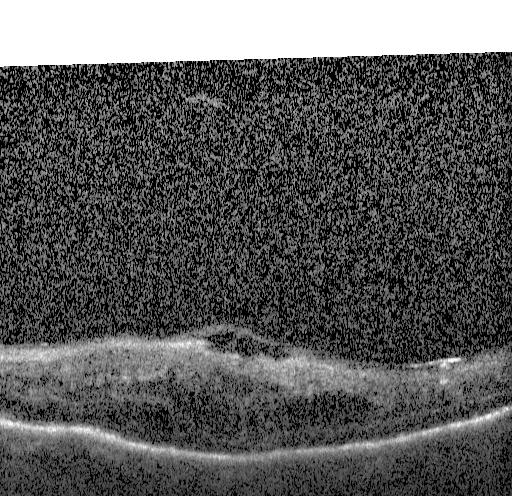
Macular scan · SD-OCT · optical coherence tomography B-scan · acquired on a Heidelberg Spectralis.
Dx: DME.